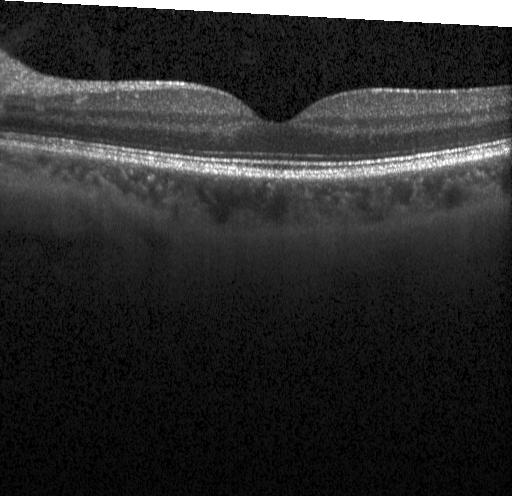

Retinal OCT B-scan · spectral-domain optical coherence tomography · through the macula. OCT finding: no choroidal neovascularization, diabetic macular edema, or drusen.